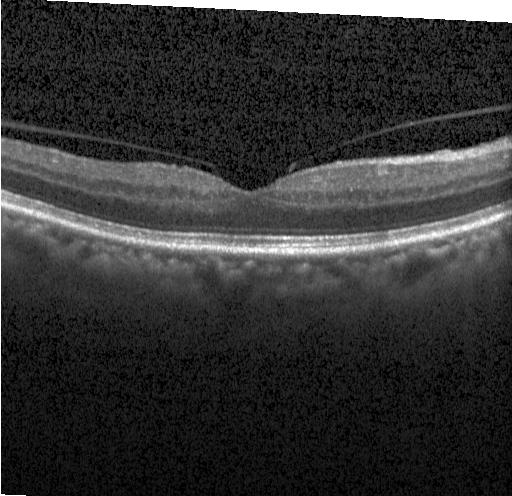
Impression: no CNV, no DME, and no drusen.